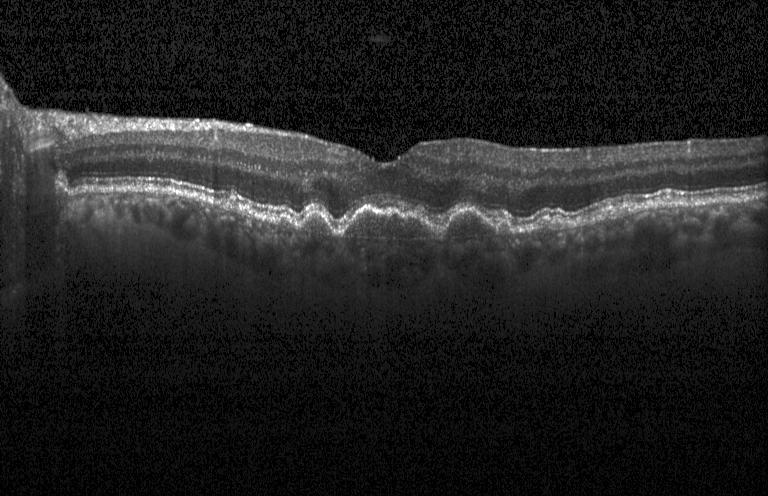 Optical coherence tomography scan. Macular OCT: sub-RPE drusenoid deposits.